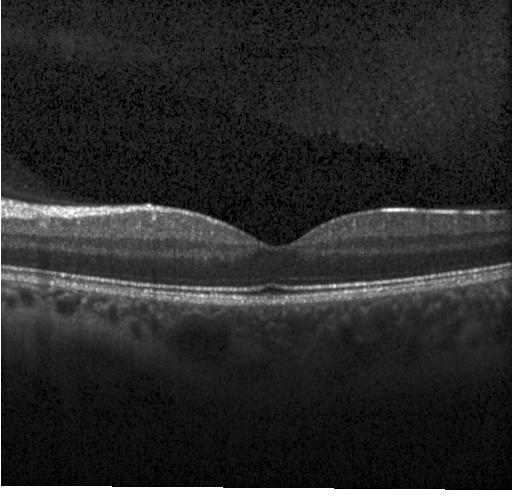 Optical coherence tomography B-scan, spectral-domain OCT
The scan shows no evidence of choroidal neovascularization, diabetic macular edema, or drusen.